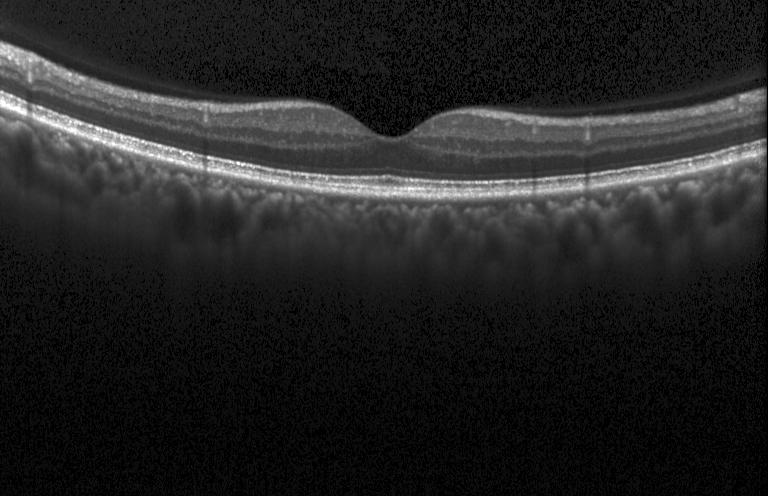

Assessment: no evidence of choroidal neovascularization, diabetic macular edema, or drusen.